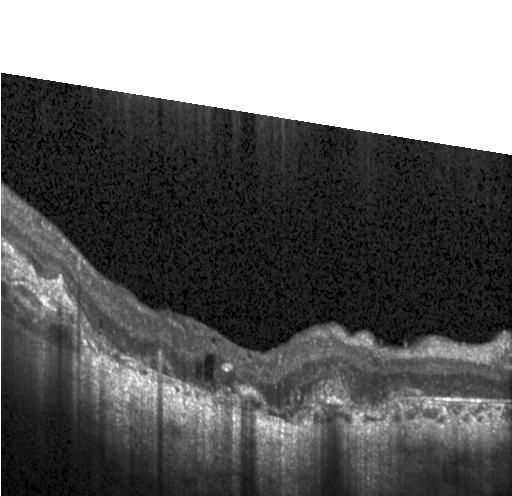
Spectral-domain OCT, retinal OCT B-scan
Assessment: choroidal neovascularization (CNV).